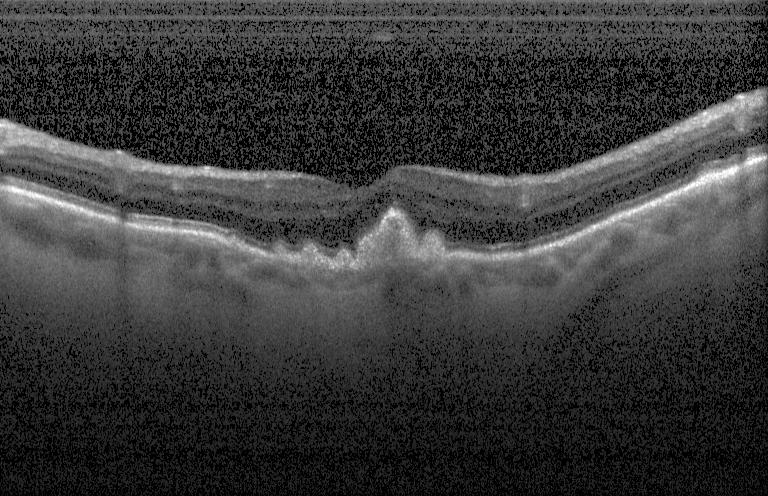
OCT B-scan. Through the macula. SD-OCT. Acquired on a Heidelberg Spectralis. This B-scan demonstrates drusen.